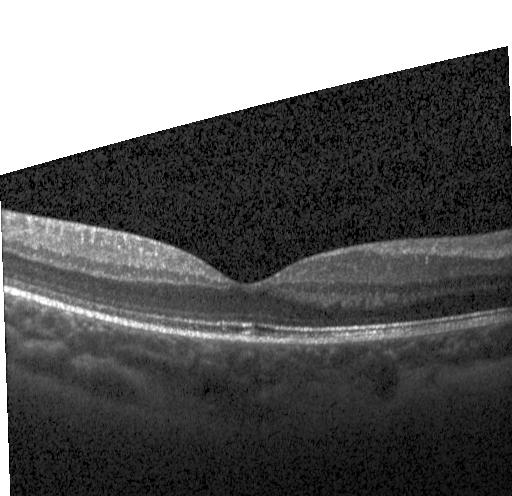

Retinal OCT B-scan — Diagnosis: neither choroidal neovascularization, diabetic macular edema, nor drusen.